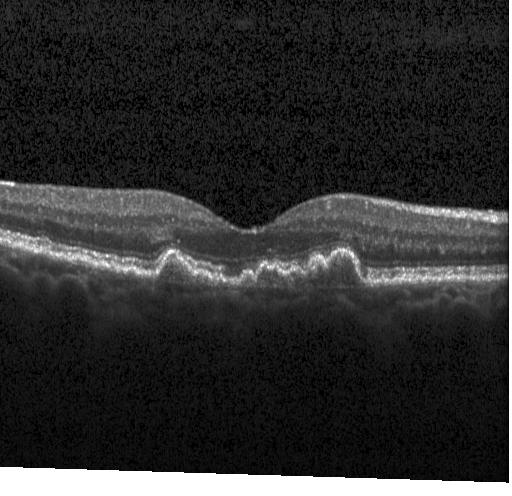
Diagnosis: drusen.